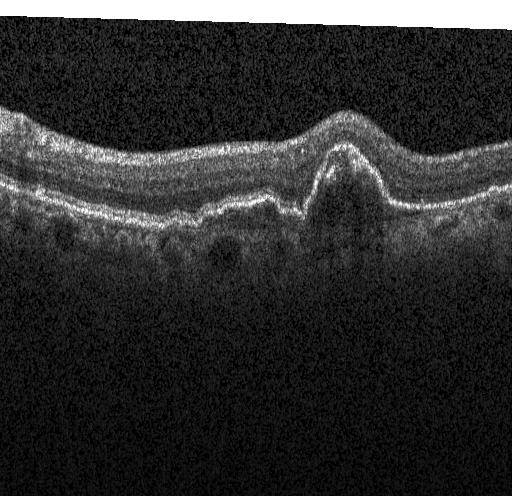 OCT B-scan
Impression: choroidal neovascularization (CNV).